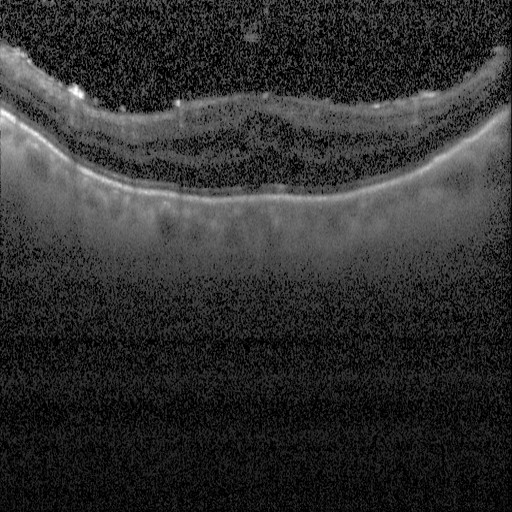
Retinal OCT cross-section. Macular OCT: diabetic macular edema.